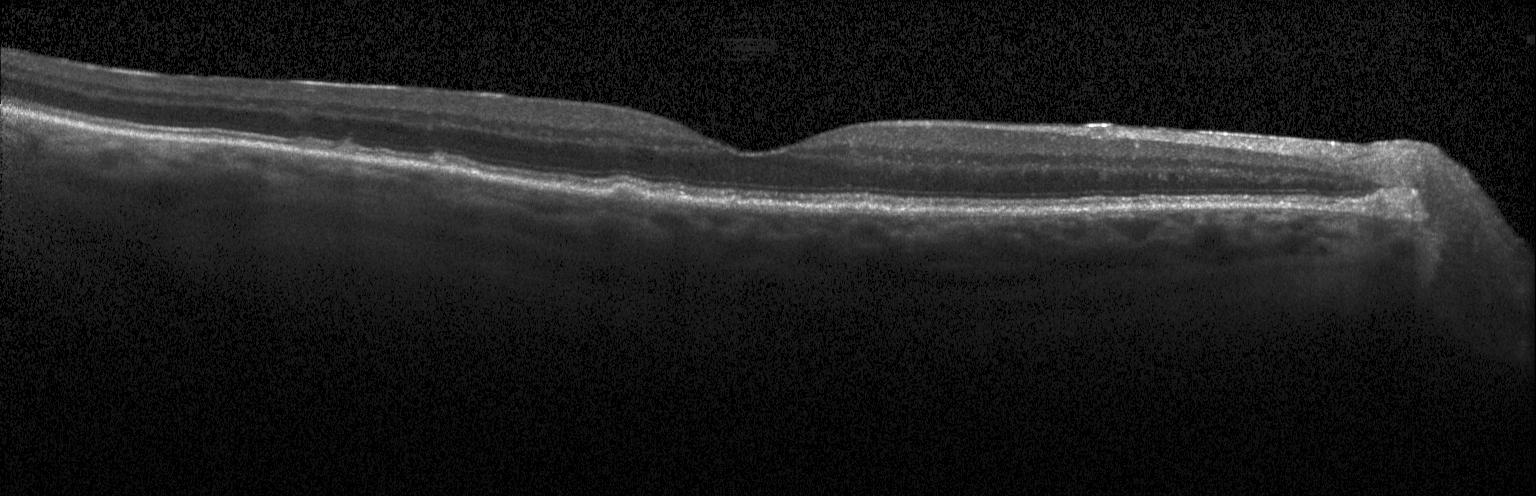 OCT B-scan. Horizontal scan through the fovea. Instrument: Heidelberg Spectralis. Spectral-domain OCT
OCT finding: sub-RPE drusenoid deposits.